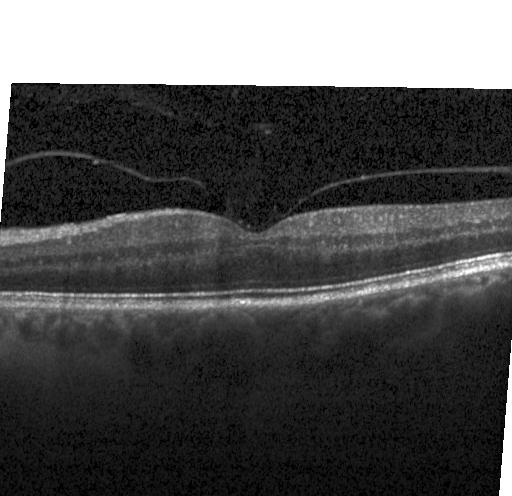

OCT line scan — The scan shows no evidence of choroidal neovascularization, diabetic macular edema, or drusen.